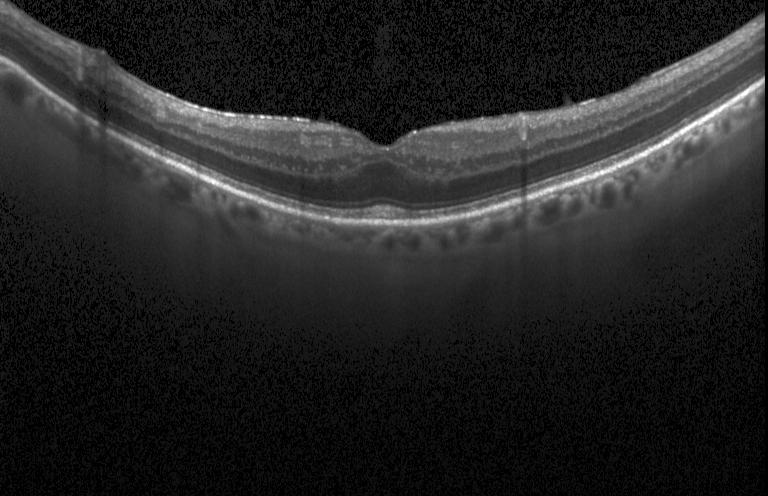

Macular scan. Retinal OCT B-scan. Spectral-domain optical coherence tomography. Heidelberg Spectralis. Diagnosis: no choroidal neovascularization, no diabetic macular edema, and no drusen.